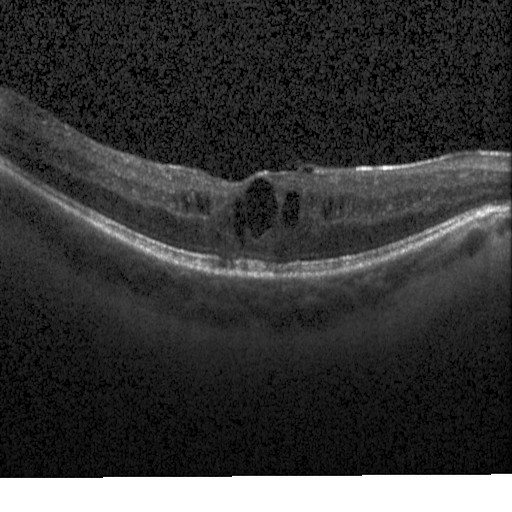 OCT B-scan showing diabetic macular edema (DME).